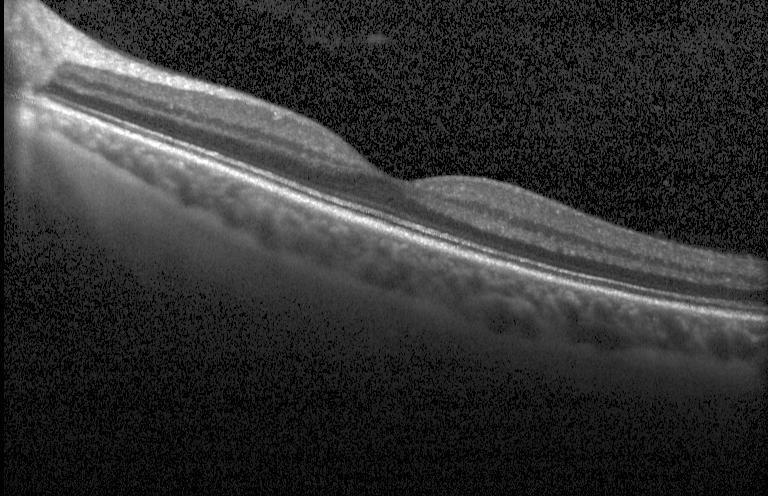 Macular scan. Instrument: Heidelberg Spectralis. Spectral-domain OCT. Retinal OCT cross-section. Finding: no evidence of choroidal neovascularization, diabetic macular edema, or drusen.